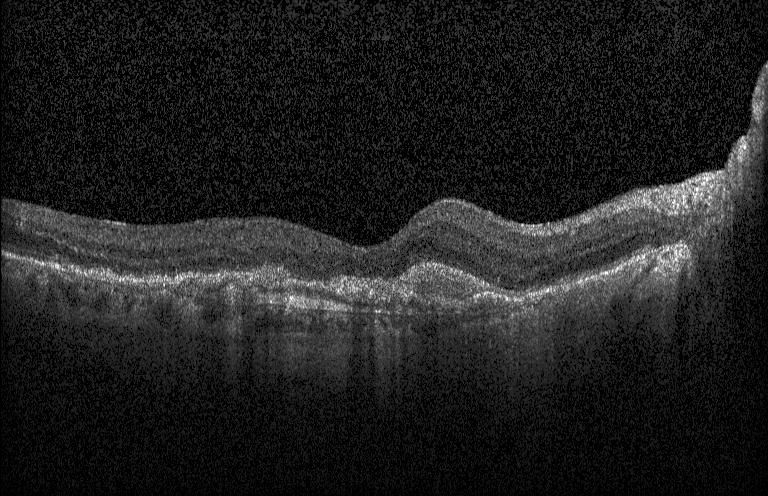

Assessment: choroidal neovascularization (CNV).